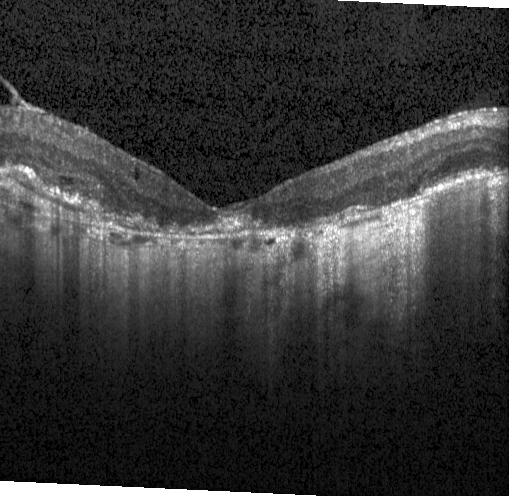
Heidelberg Spectralis OCT system; retinal OCT cross-section; spectral-domain optical coherence tomography
The scan shows a choroidal neovascular membrane.